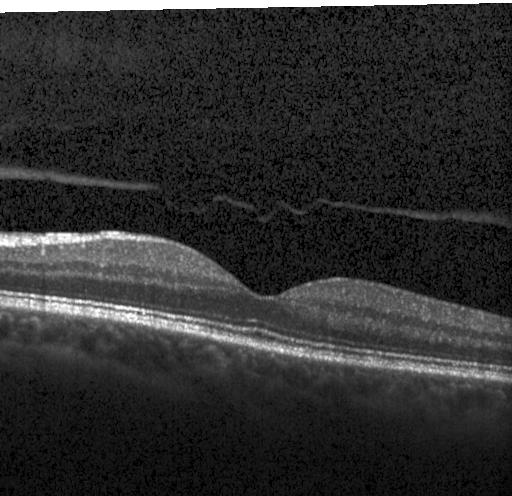
OCT B-scan showing no choroidal neovascularization, diabetic macular edema, or drusen.